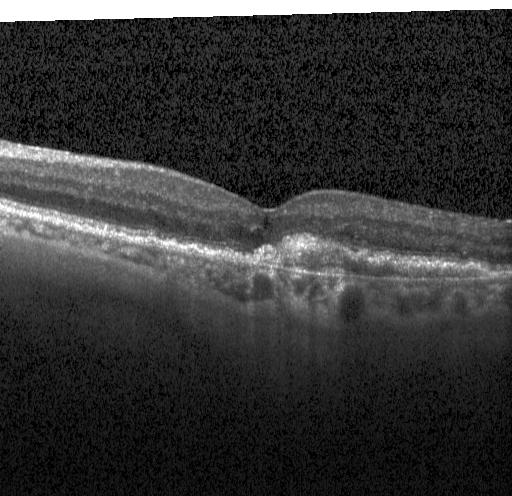 Through the macula · OCT B-scan
Macular OCT: choroidal neovascularization.